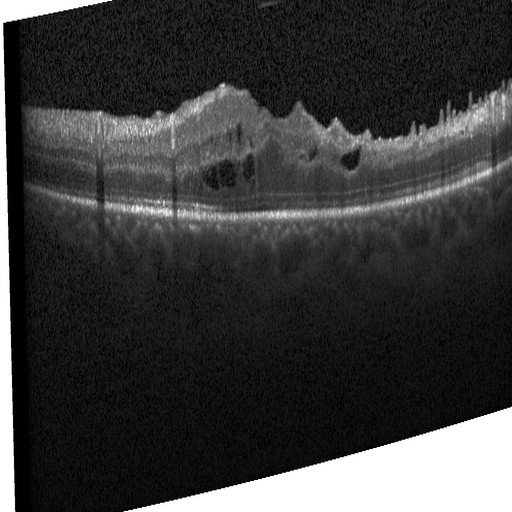 OCT B-scan, through the macula, spectral-domain OCT — Dx: diabetic macular edema.